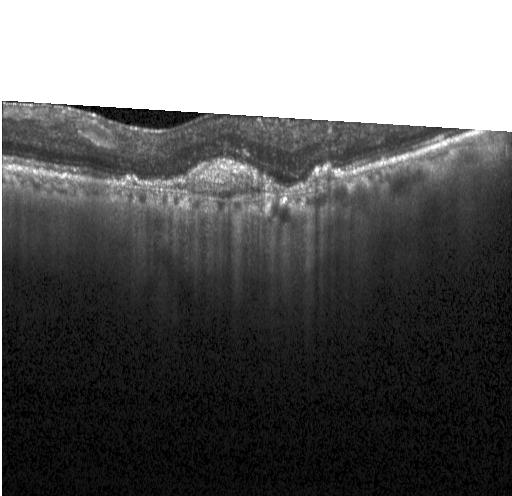

OCT B-scan showing CNV.